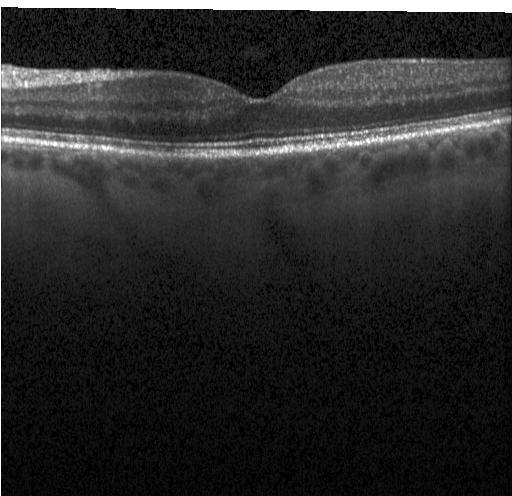 Assessment: no choroidal neovascularization, no diabetic macular edema, and no drusen.